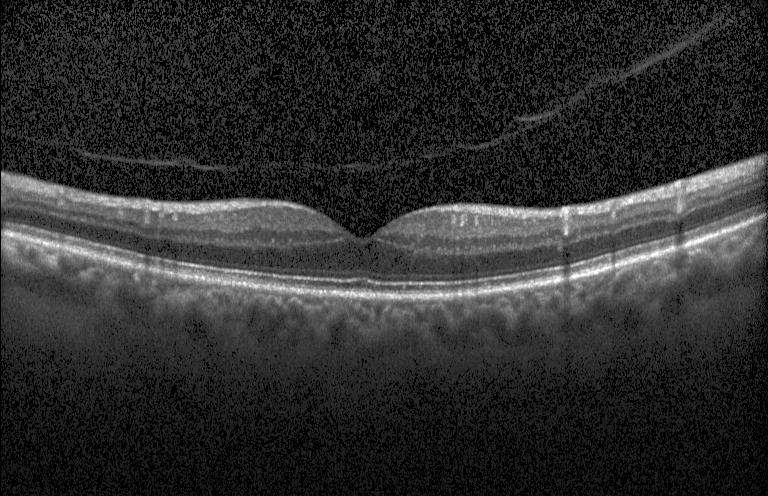

OCT B-scan — Impression: neither CNV, DME, nor drusen.